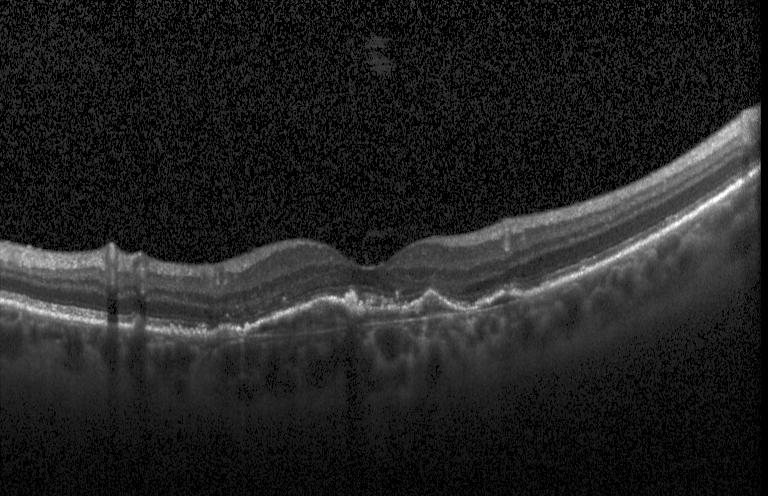

Diagnosis: CNV.